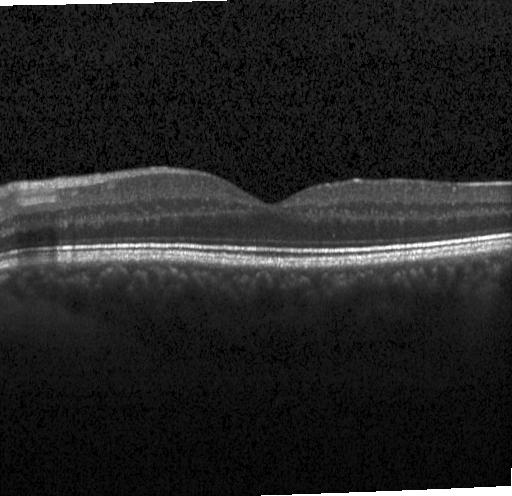

Impression: neither choroidal neovascularization, diabetic macular edema, nor drusen.